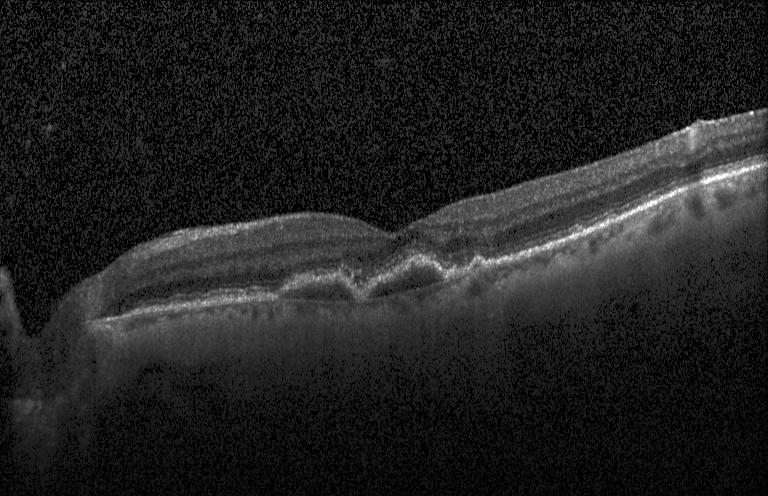

Impression: choroidal neovascularization.